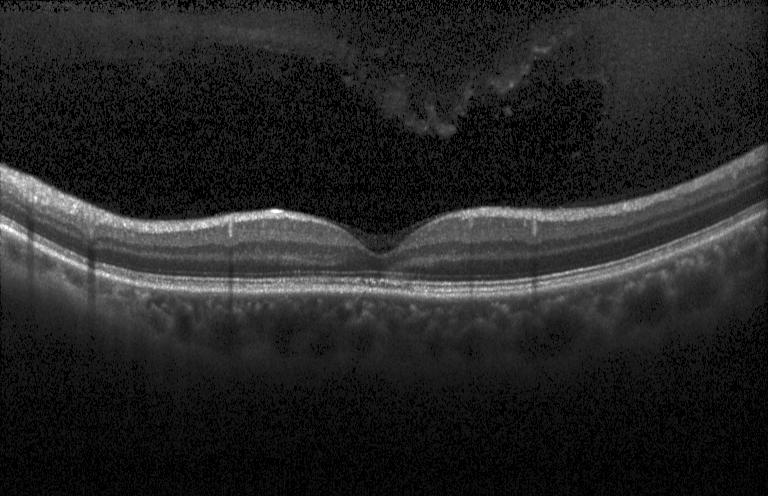
Optical coherence tomography B-scan, through the macula, spectral-domain OCT. Diagnosis: neither choroidal neovascularization, diabetic macular edema, nor drusen.